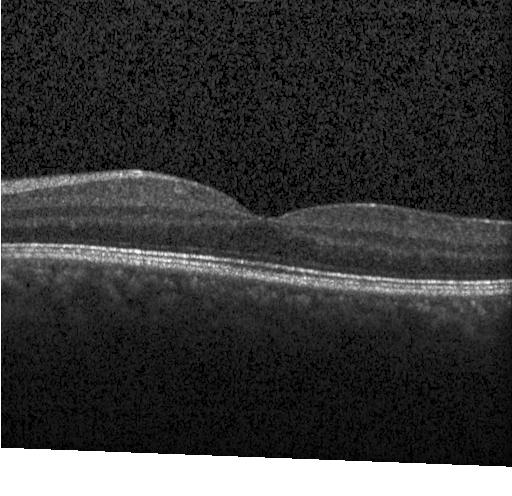 OCT scan showing no choroidal neovascularization, no diabetic macular edema, and no drusen.